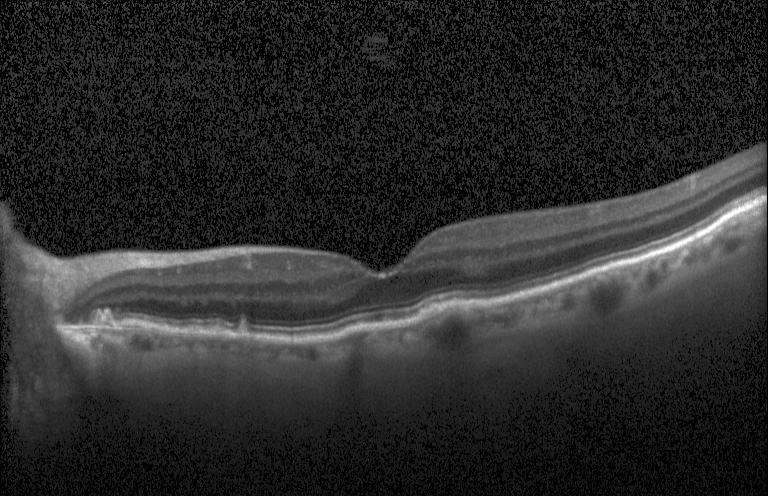 Optical coherence tomography scan · SD-OCT · macular scan · instrument: Heidelberg Spectralis.
Macular OCT: sub-RPE drusenoid deposits.